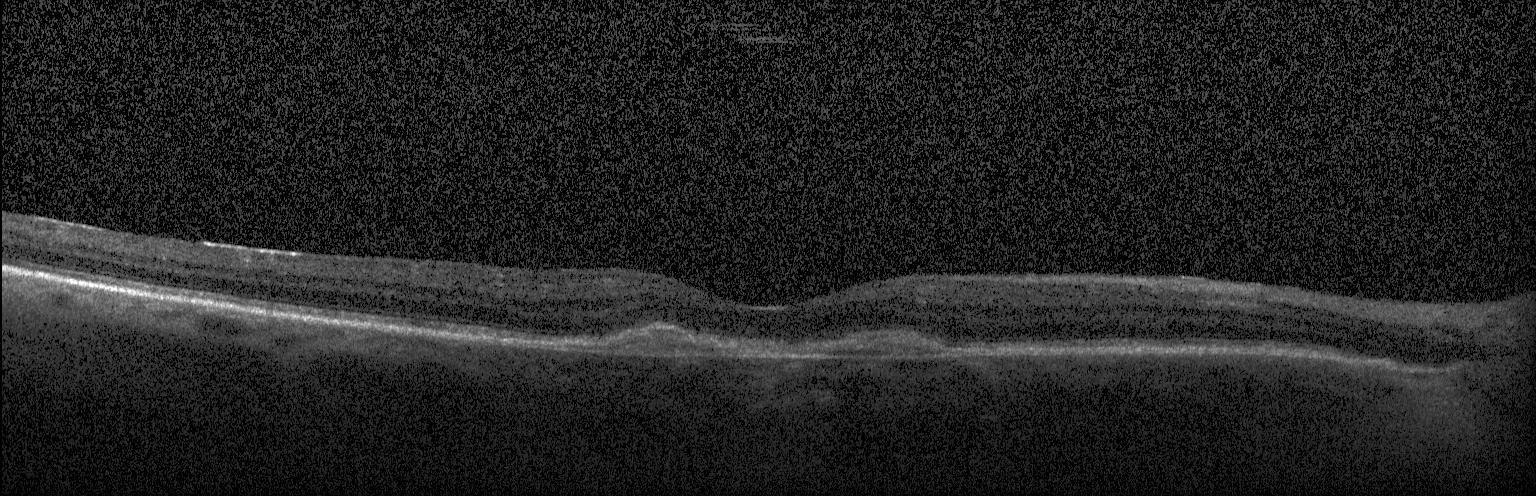
Retinal OCT B-scan; macular scan; Heidelberg Spectralis
Diagnosis: choroidal neovascularization (CNV).